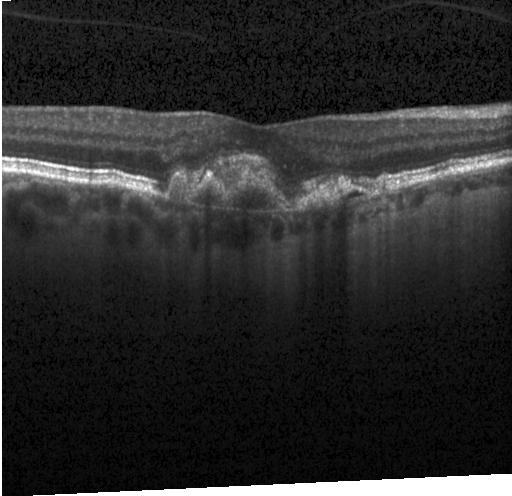

Optical coherence tomography B-scan
Diagnosis: CNV.